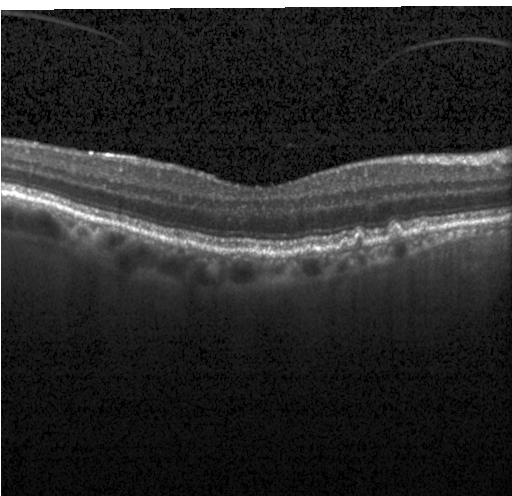

Macular scan · retinal OCT cross-section. Impression: drusen.